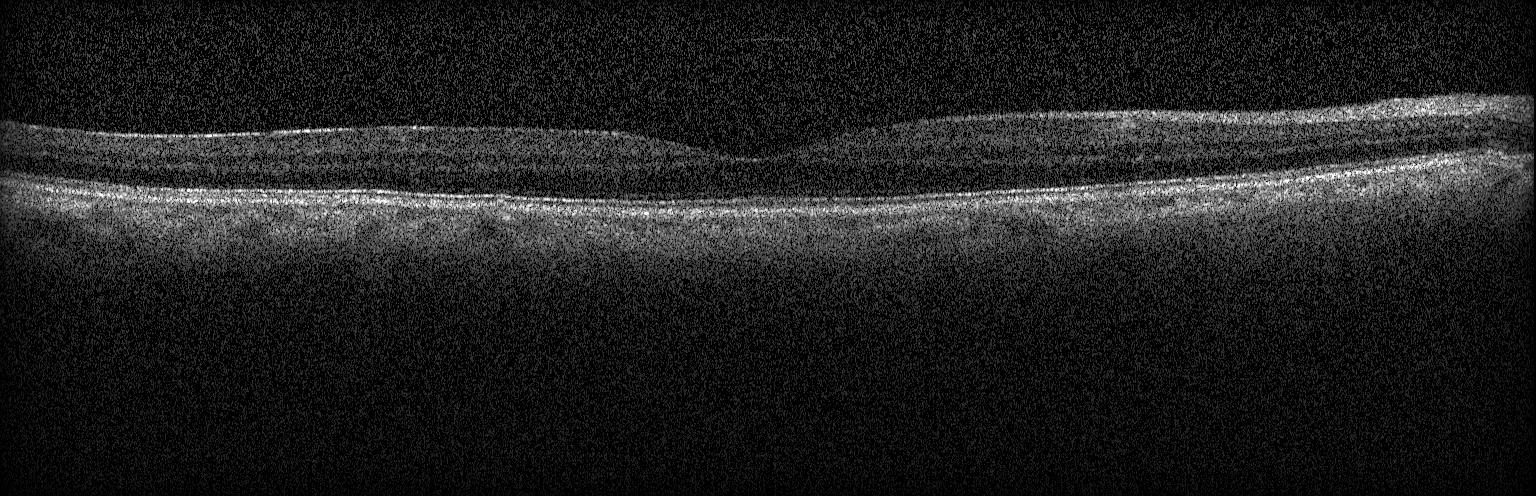
Finding: no choroidal neovascularization, diabetic macular edema, or drusen.